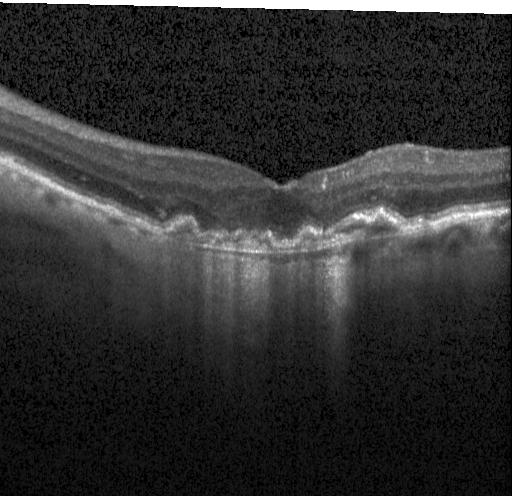
Finding: choroidal neovascularization.